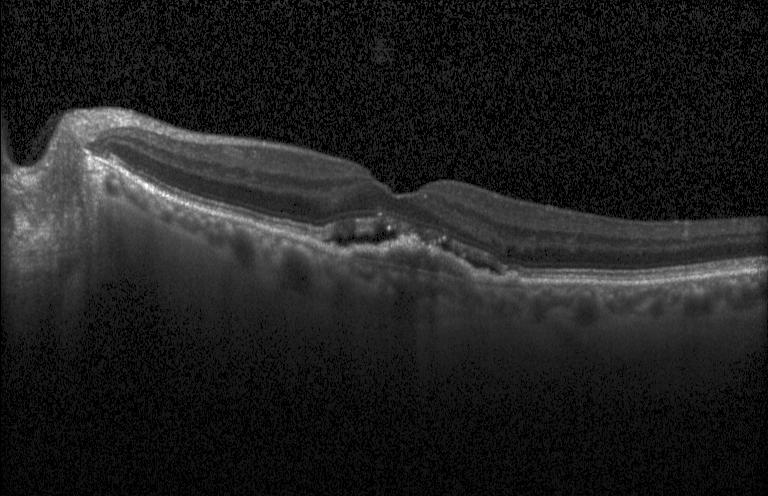
Impression: choroidal neovascularization (CNV).